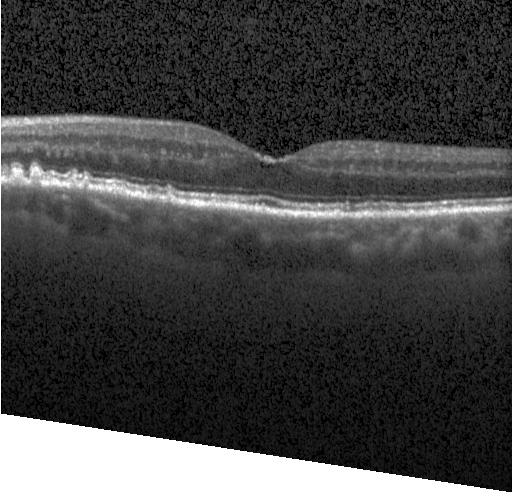 Heidelberg Spectralis OCT system. Spectral-domain OCT. Through the macula. Optical coherence tomography B-scan.
Assessment: multiple drusen.